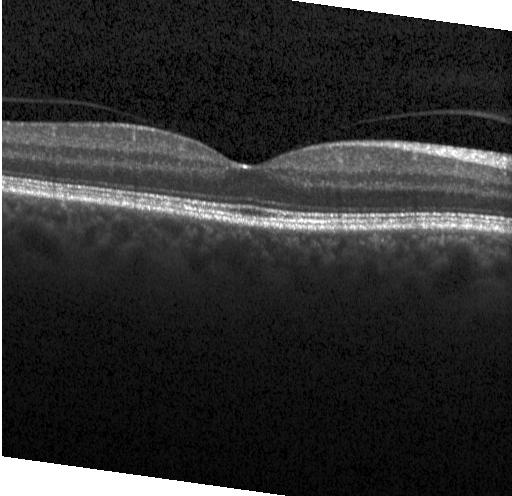

Diagnosis: no CNV, no DME, and no drusen.